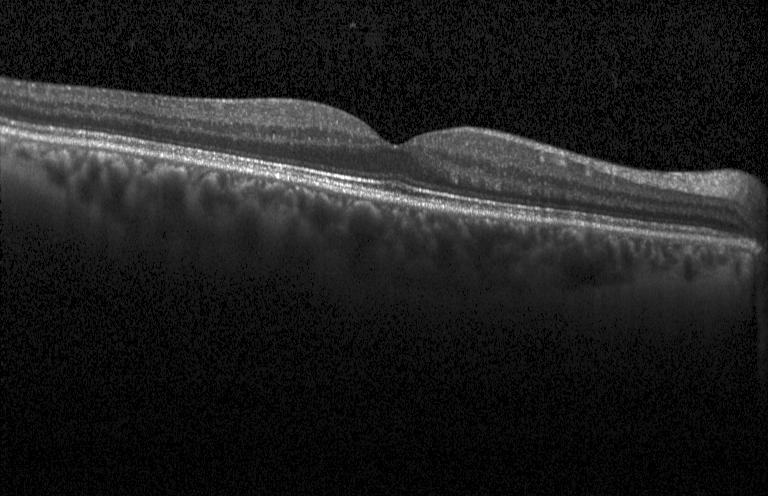 Through the macula. Spectral-domain optical coherence tomography. Optical coherence tomography B-scan. Heidelberg Spectralis
Dx: no CNV, no DME, and no drusen.